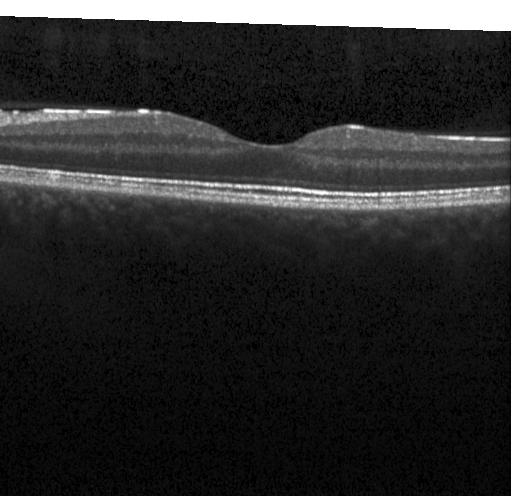
OCT B-scan showing neither CNV, DME, nor drusen.